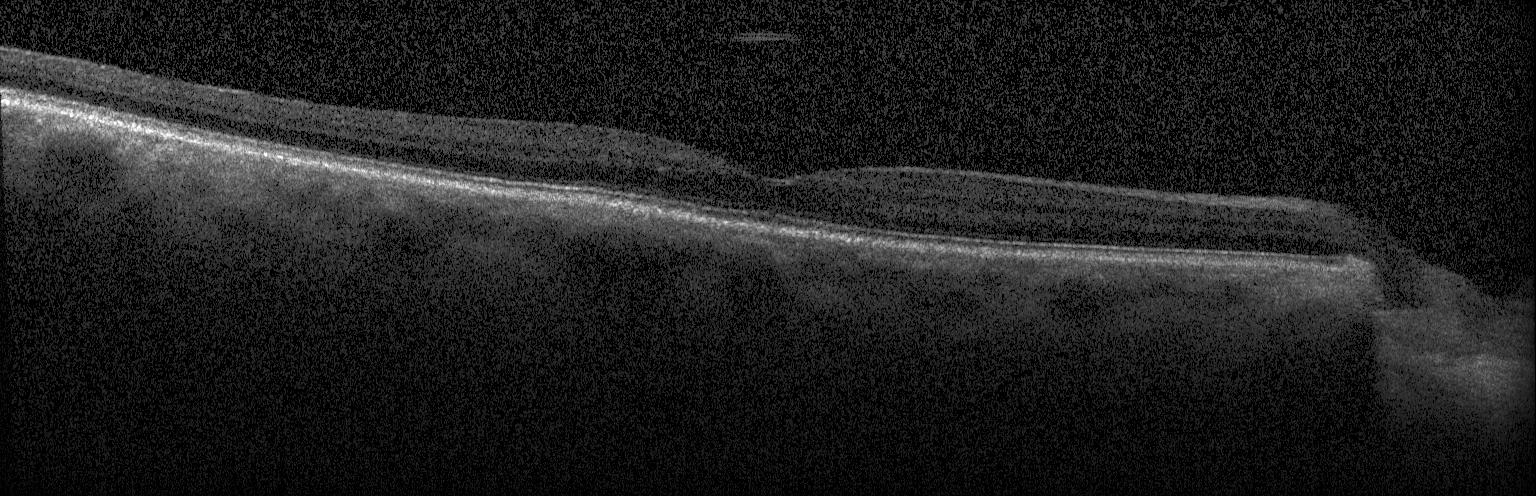
OCT line scan · SD-OCT
No choroidal neovascularization, no diabetic macular edema, and no drusen.